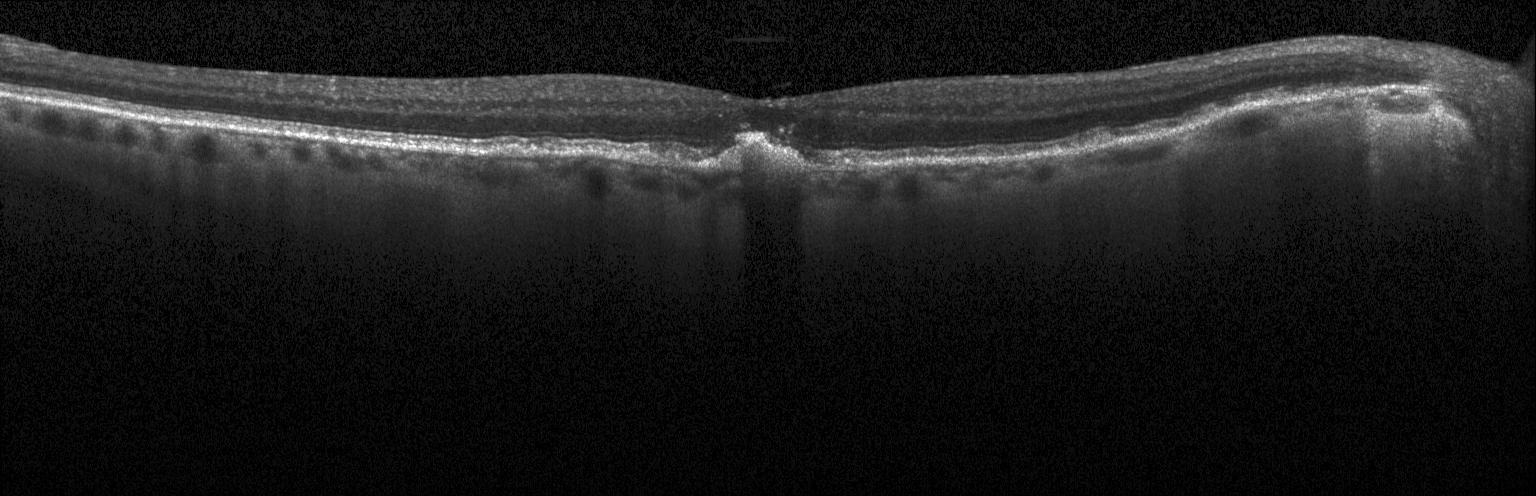 OCT line scan.
Finding: multiple drusen.